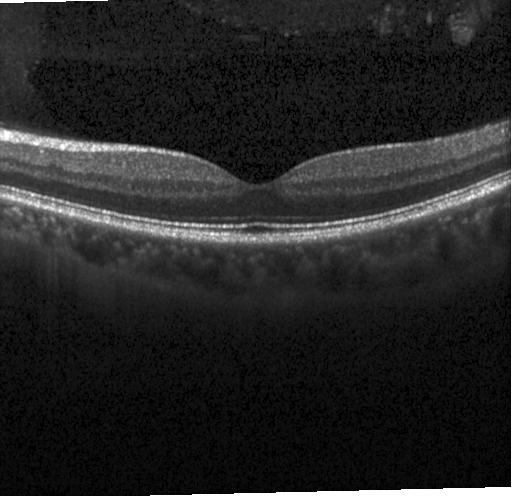
Spectral-domain OCT · optical coherence tomography B-scan · fovea-centered — The scan shows no choroidal neovascularization, diabetic macular edema, or drusen.